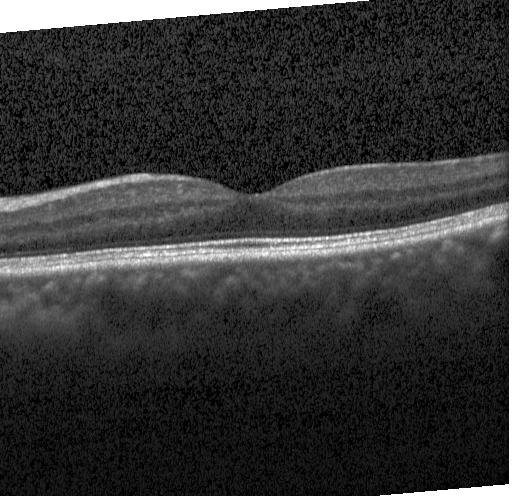 Diagnosis: no evidence of choroidal neovascularization, diabetic macular edema, or drusen.